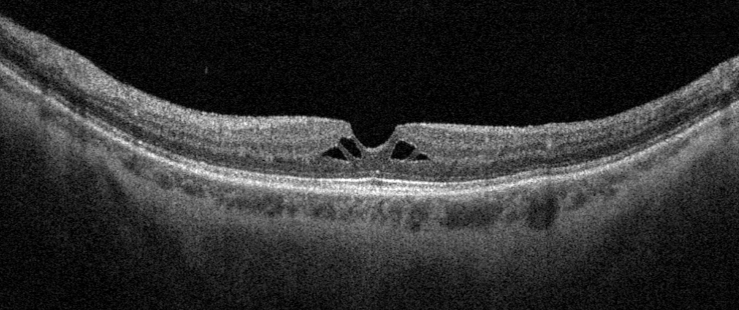 Acquired on an Optovue Avanti RTVue XR · optical coherence tomography scan.
The scan shows VID.